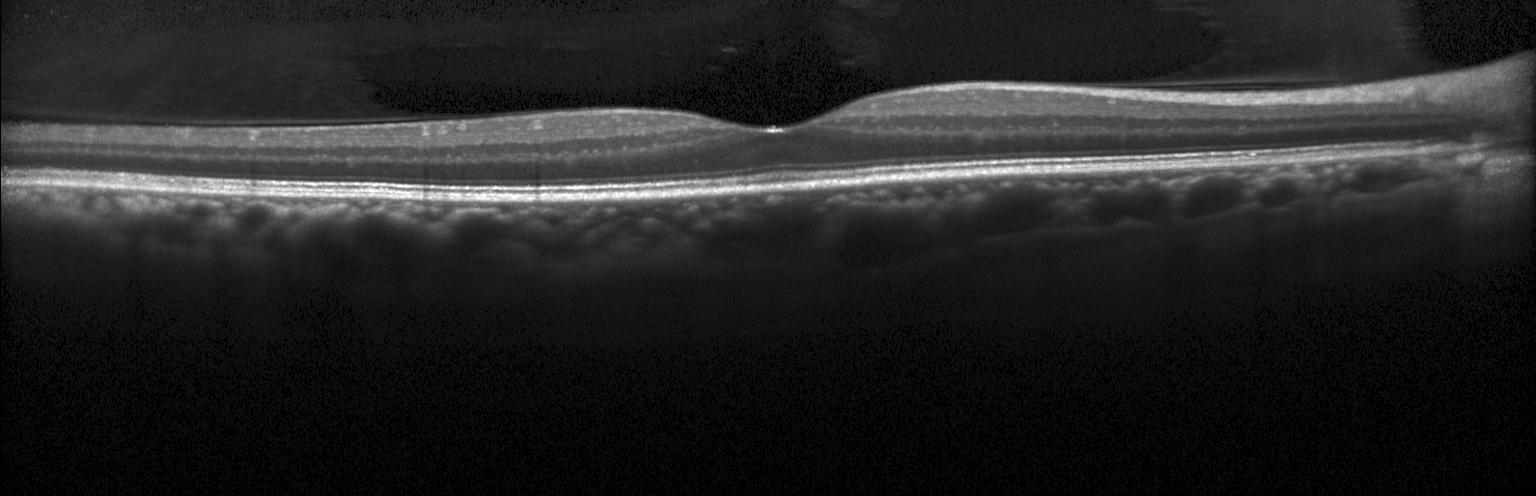 Finding: no choroidal neovascularization, no diabetic macular edema, and no drusen.